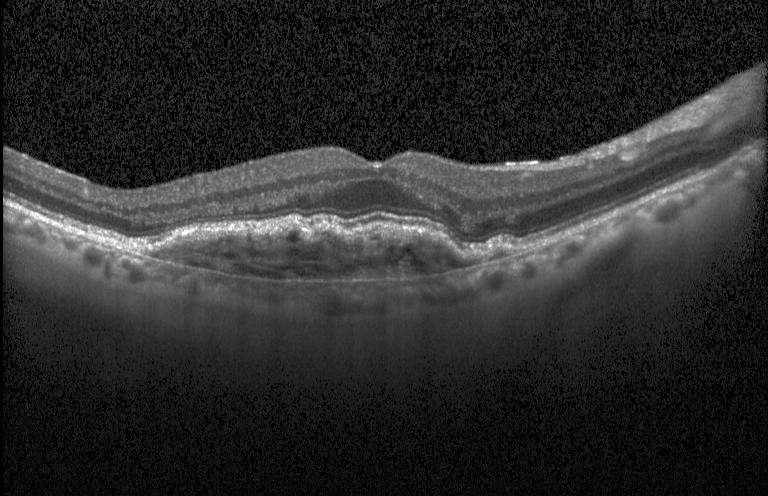 SD-OCT; optical coherence tomography B-scan. Diagnosis: a choroidal neovascular membrane.